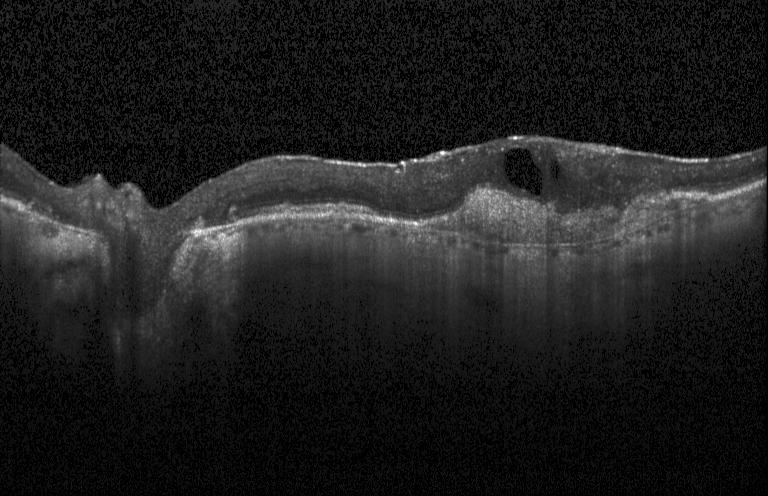

Macular OCT: CNV.